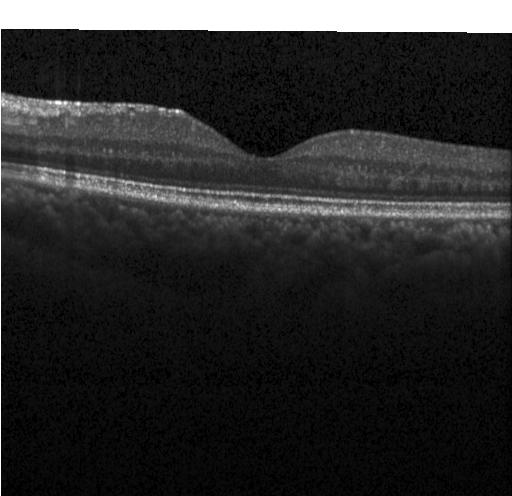

Spectral-domain optical coherence tomography; optical coherence tomography scan.
Diagnosis: no evidence of CNV, DME, or drusen.